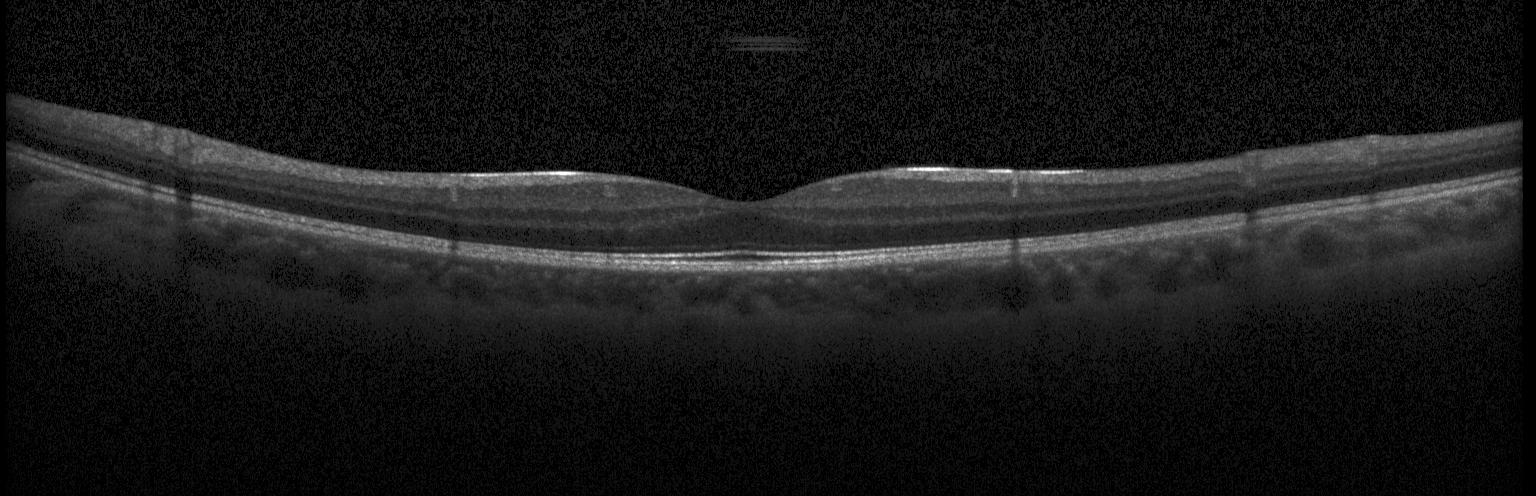
Instrument: Heidelberg Spectralis; SD-OCT; OCT B-scan; macular scan. This B-scan demonstrates no choroidal neovascularization, diabetic macular edema, or drusen.